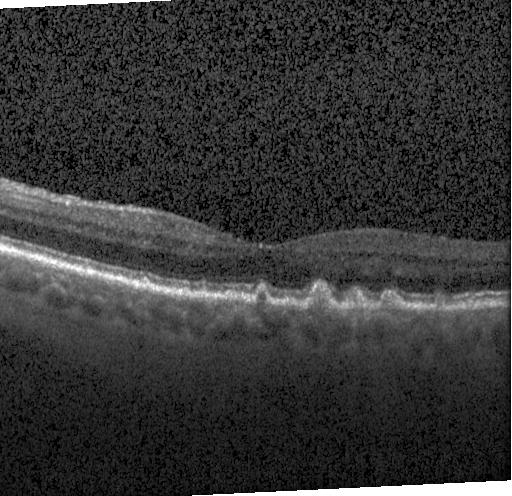
Heidelberg Spectralis, OCT line scan.
Finding: drusen.